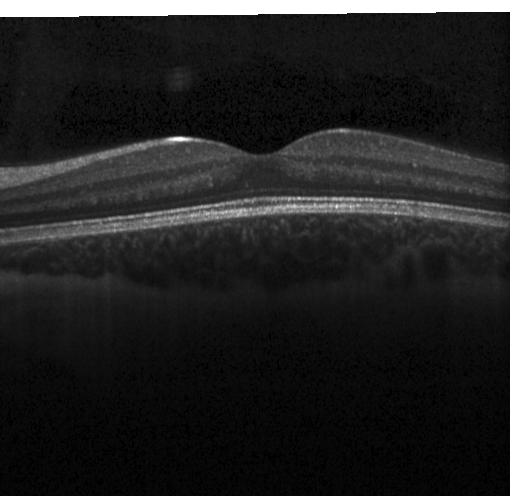 Heidelberg Spectralis; macular scan; retinal OCT B-scan; SD-OCT. Assessment: no evidence of CNV, DME, or drusen.